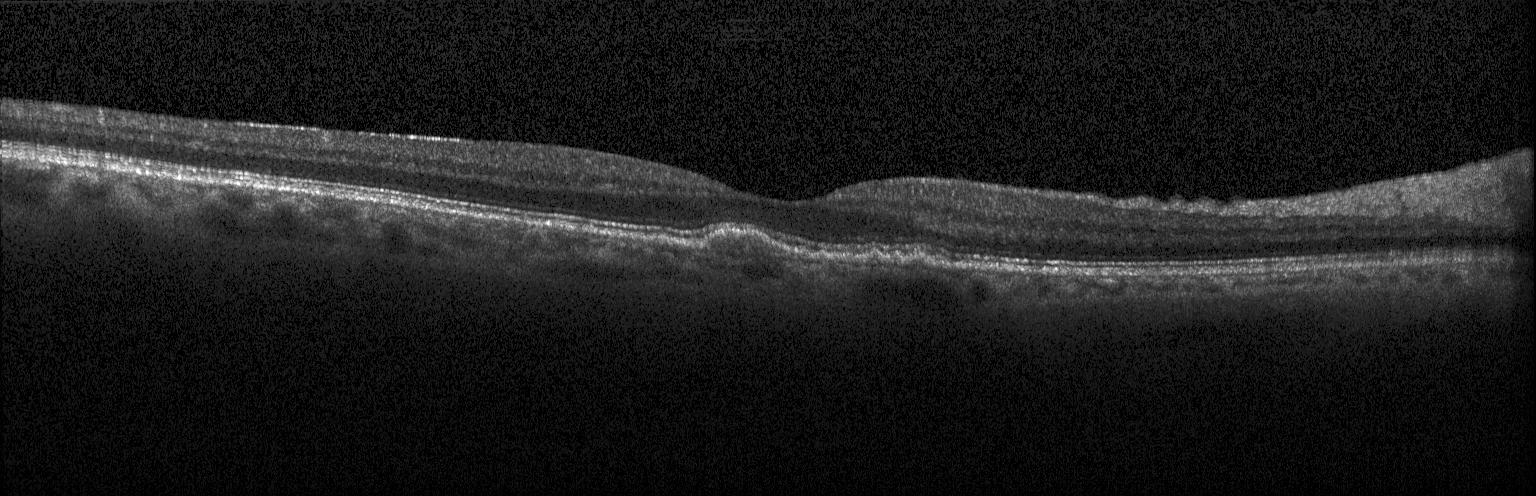
Assessment: multiple drusen.